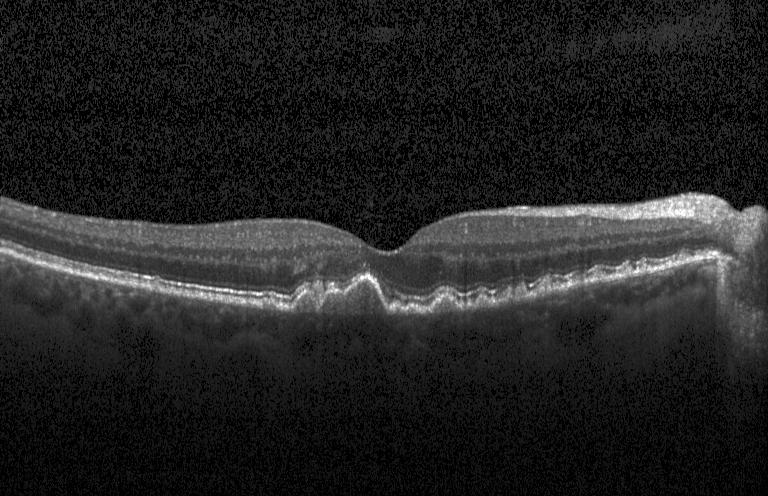
Fovea-centered. Heidelberg Spectralis OCT system. Retinal OCT cross-section
Finding: sub-RPE drusenoid deposits.